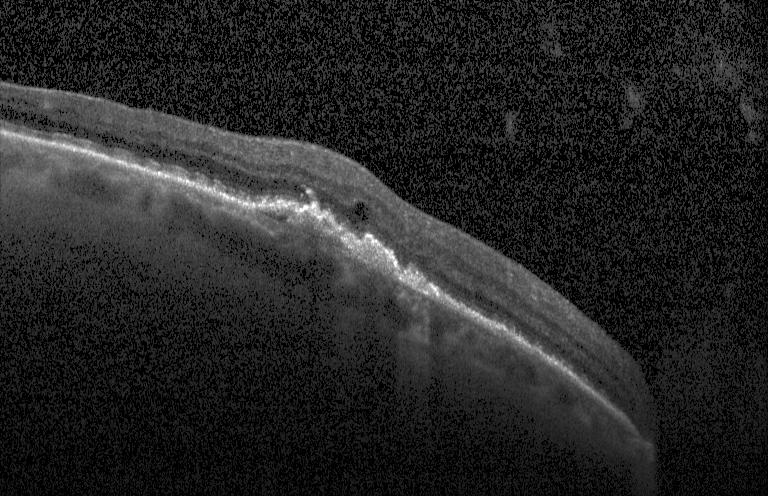
Retinal OCT cross-section; horizontal scan through the fovea
Diagnosis: CNV.